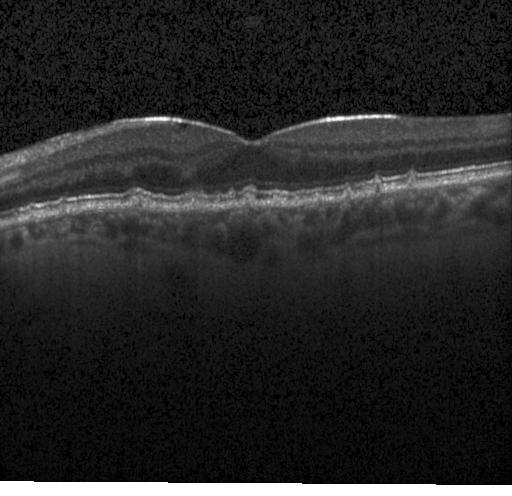

Spectral-domain optical coherence tomography. Heidelberg Spectralis OCT system. Optical coherence tomography scan. Finding: drusen.